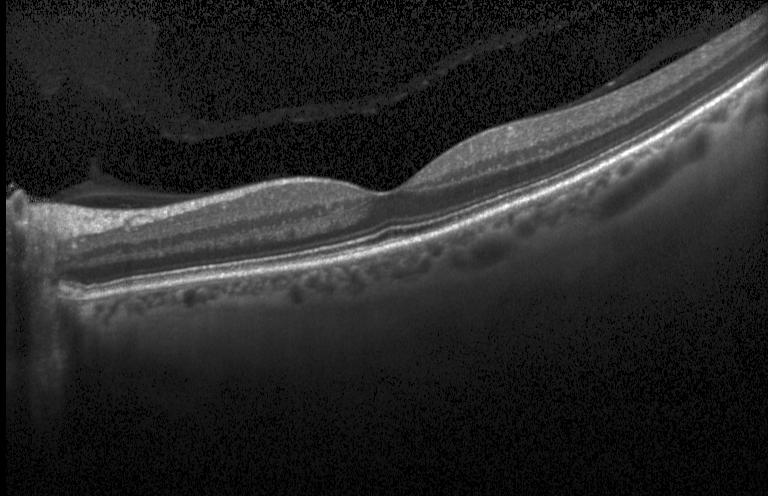

Spectral-domain OCT; macular scan; retinal OCT cross-section; instrument: Heidelberg Spectralis.
Impression: no choroidal neovascularization, no diabetic macular edema, and no drusen.